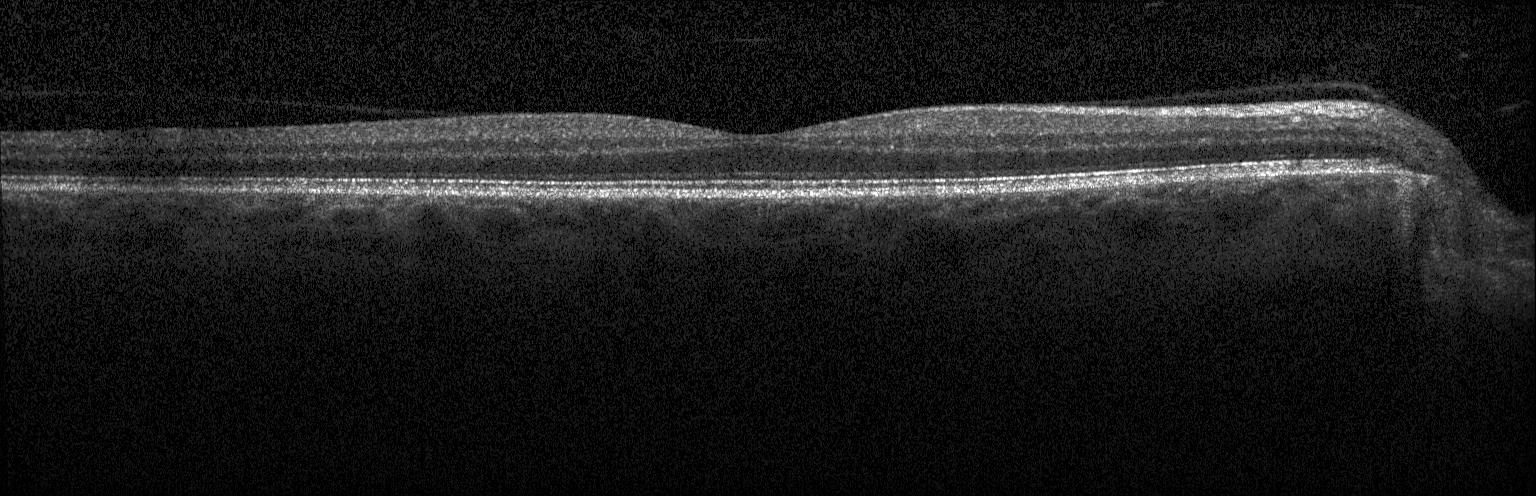
OCT line scan — Macular OCT: no choroidal neovascularization, no diabetic macular edema, and no drusen.